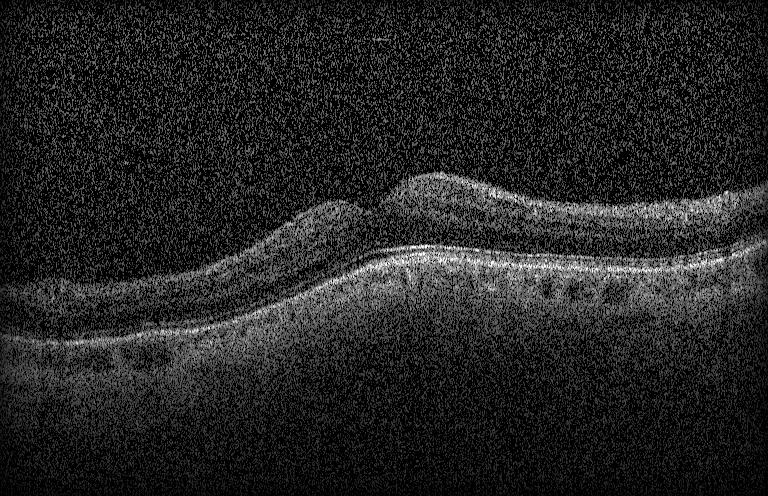

OCT line scan. Spectral-domain optical coherence tomography. Macular scan.
Diagnosis: no evidence of CNV, DME, or drusen.